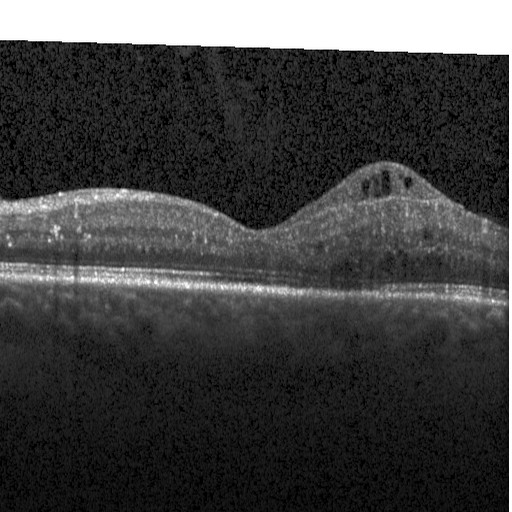 The scan shows diabetic macular edema (DME).